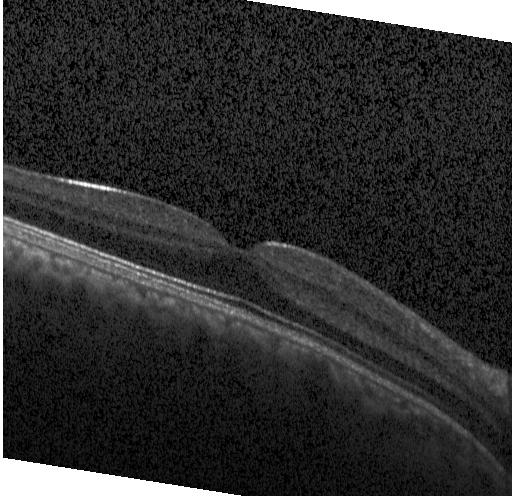 Optical coherence tomography scan; centered on the fovea.
Dx: no evidence of choroidal neovascularization, diabetic macular edema, or drusen.